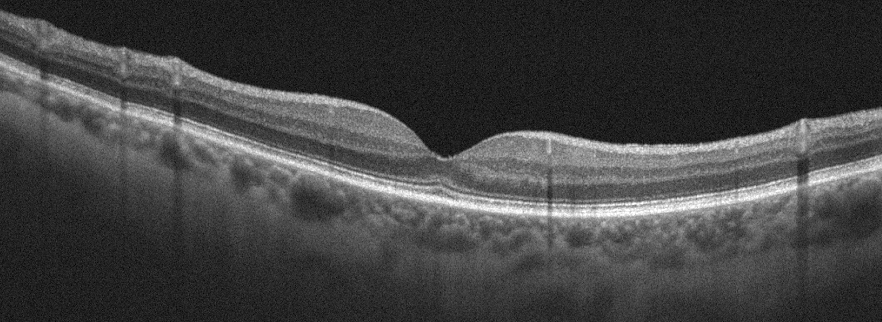
OS; retinal OCT cross-section — This B-scan demonstrates no AMD, DME, ERM, RAO, RVO, or VID.